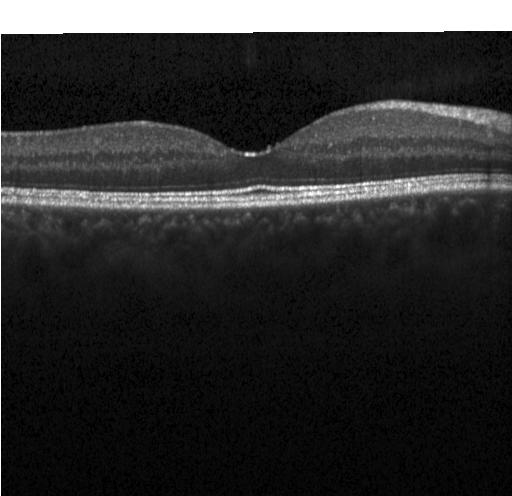

Impression: no evidence of choroidal neovascularization, diabetic macular edema, or drusen.